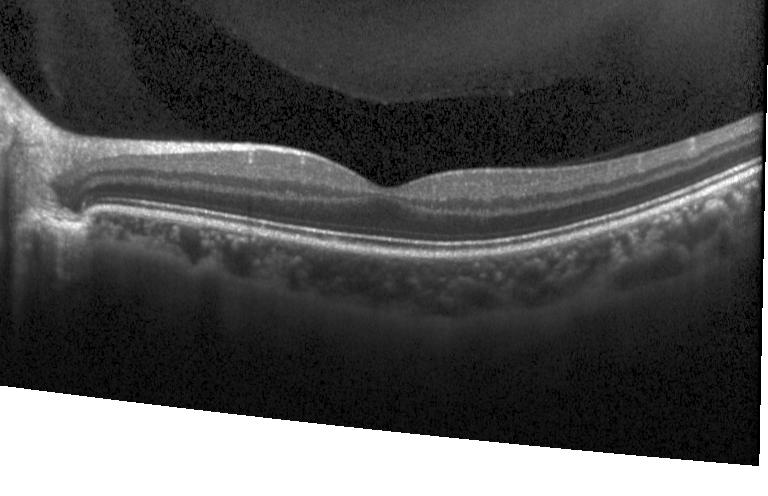 Macular OCT: no choroidal neovascularization, no diabetic macular edema, and no drusen.